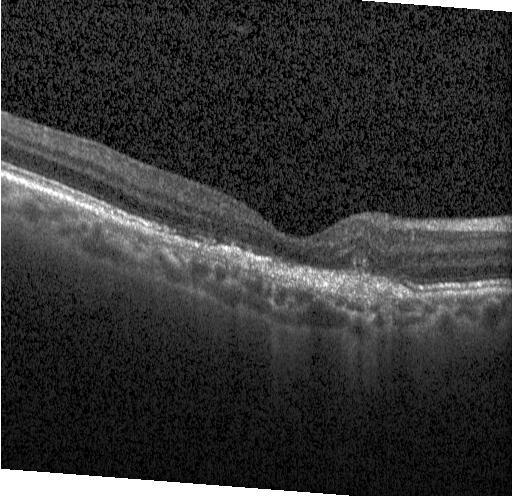

Optical coherence tomography B-scan; horizontal scan through the fovea.
Assessment: a choroidal neovascular membrane.